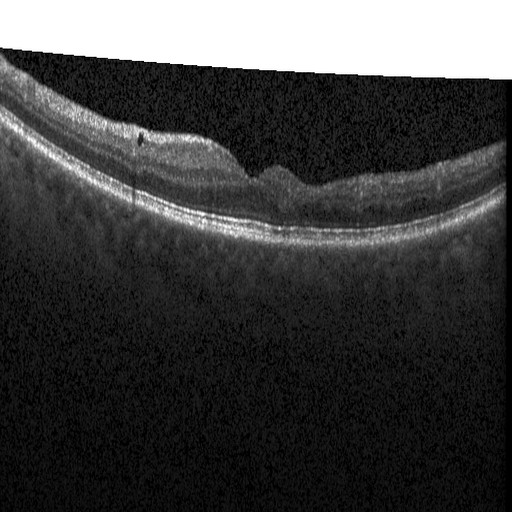

Through the macula. SD-OCT. Retinal OCT B-scan
Impression: diabetic macular edema (DME).